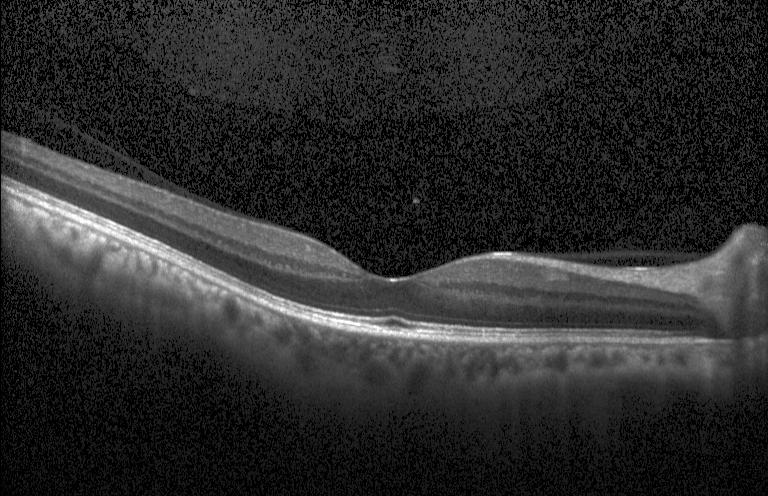
OCT B-scan
Impression: no CNV, DME, or drusen.